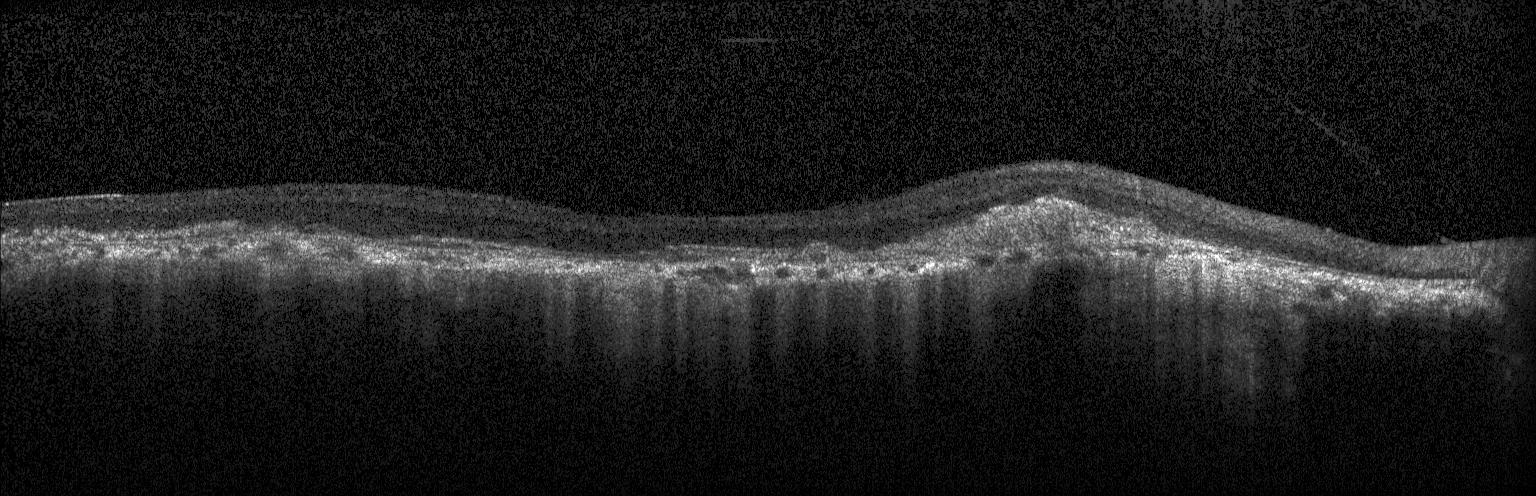

Finding: a choroidal neovascular membrane.